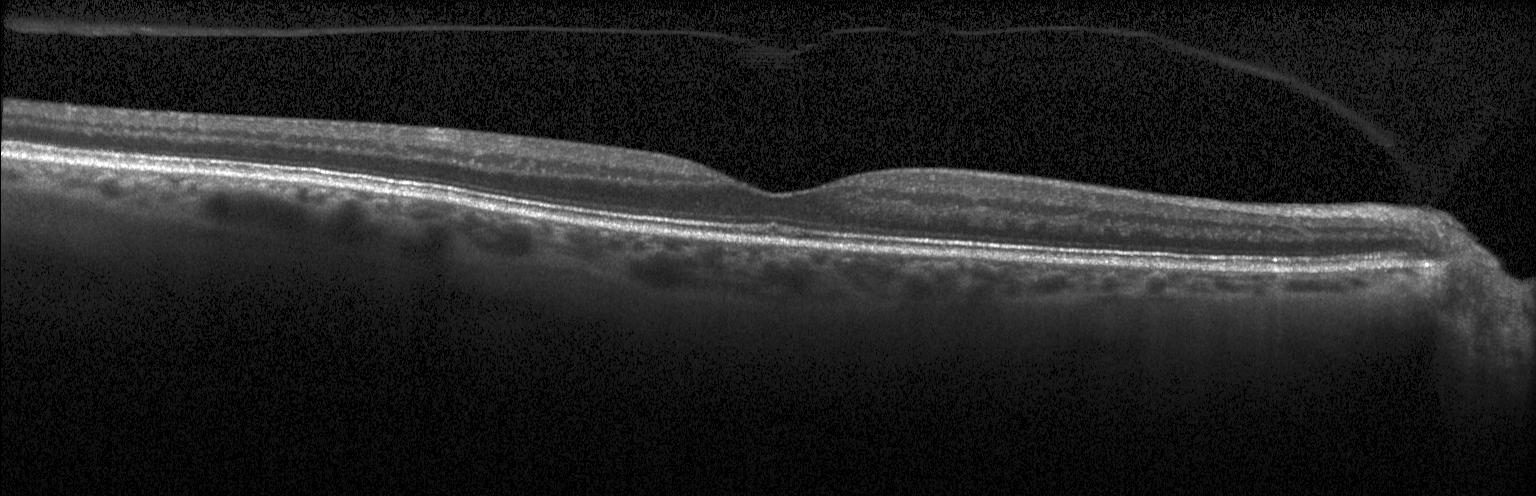

The scan shows no CNV, no DME, and no drusen.